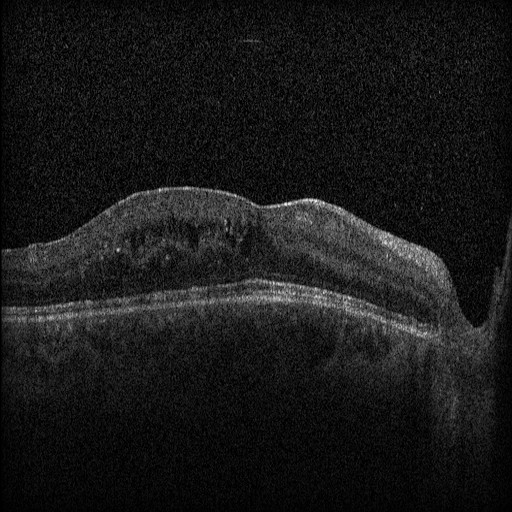 Through the macula. Optical coherence tomography scan.
This B-scan demonstrates diabetic macular edema (DME).